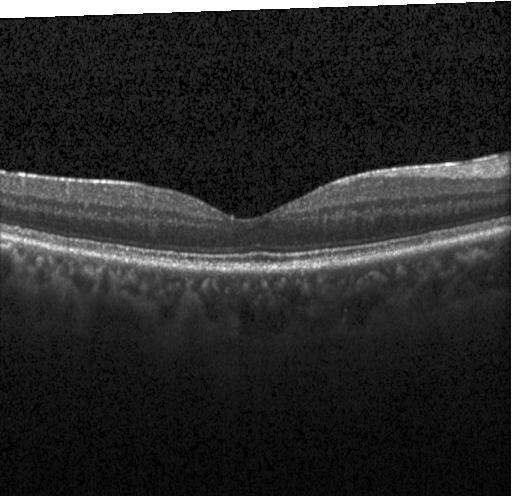

Acquired on a Heidelberg Spectralis, retinal OCT B-scan.
OCT finding: no evidence of choroidal neovascularization, diabetic macular edema, or drusen.